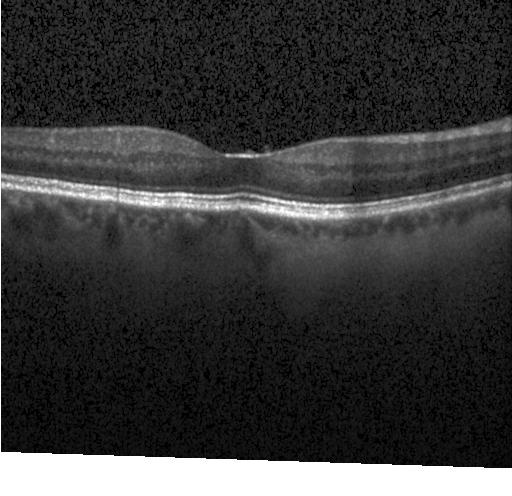
Dx: neither choroidal neovascularization, diabetic macular edema, nor drusen.